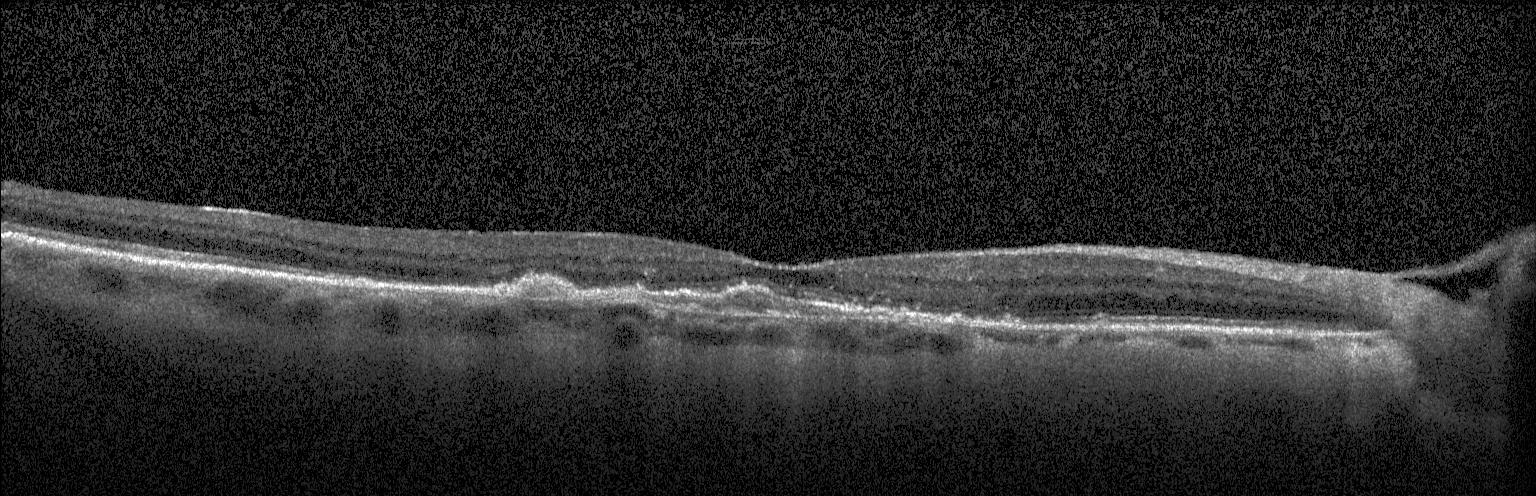
Finding: CNV.